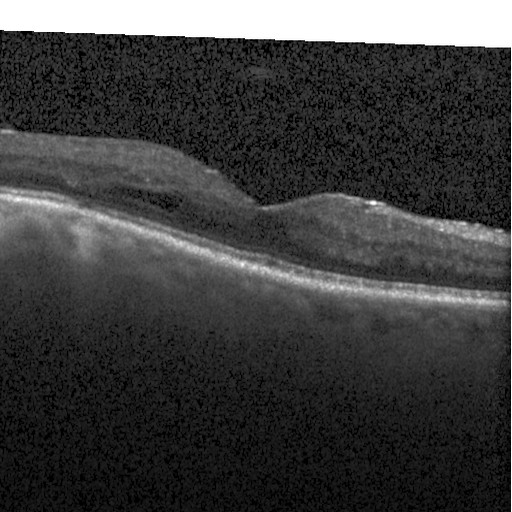

OCT line scan · centered on the fovea
DME.